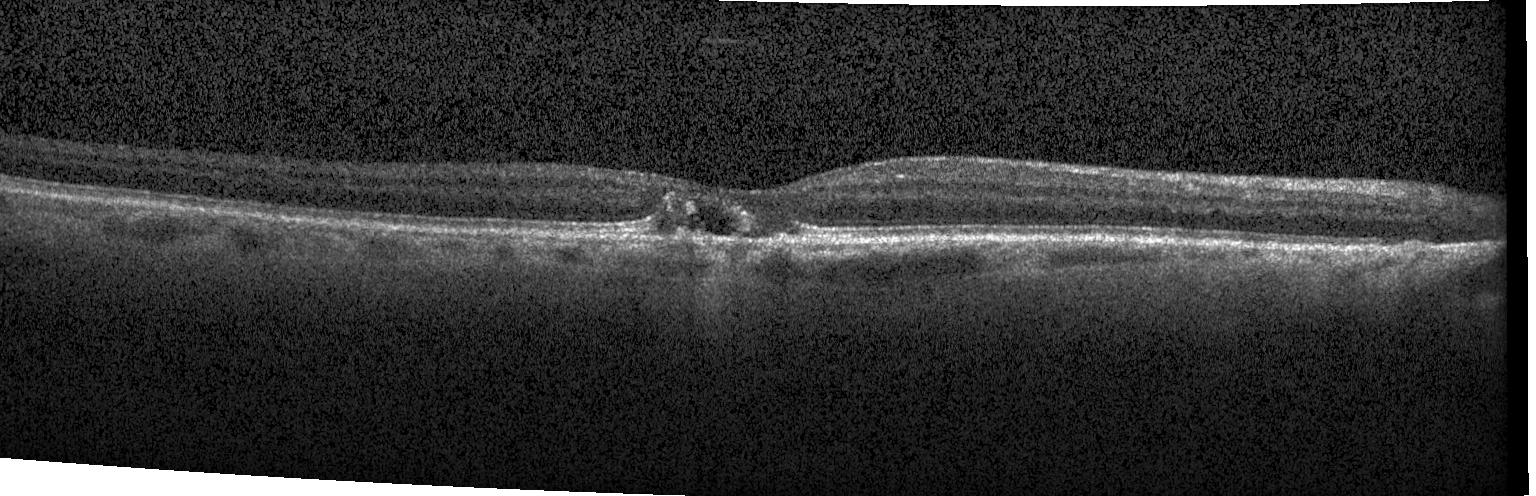

OCT B-scan · Heidelberg Spectralis · spectral-domain optical coherence tomography · through the macula
The scan shows choroidal neovascularization (CNV).